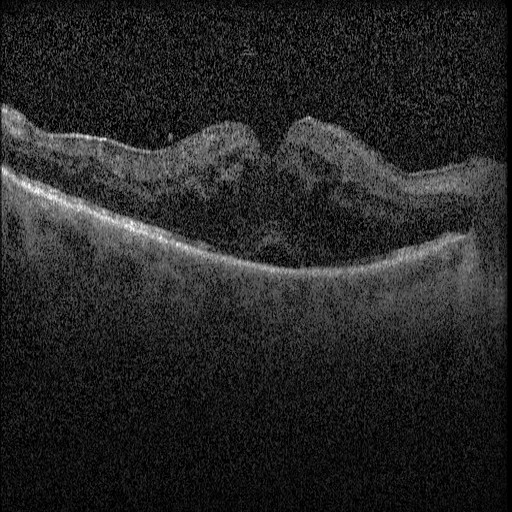
Assessment: DME.